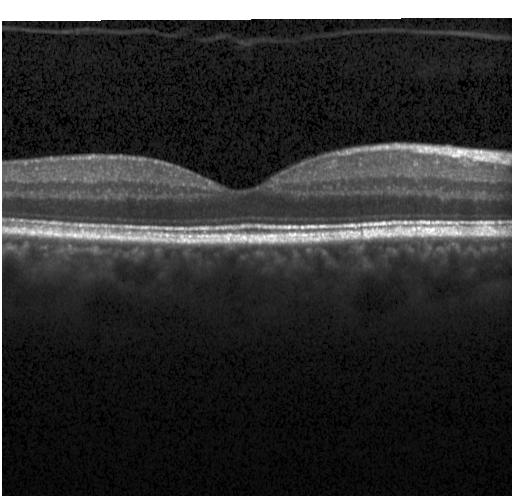
Diagnosis: no choroidal neovascularization, no diabetic macular edema, and no drusen.